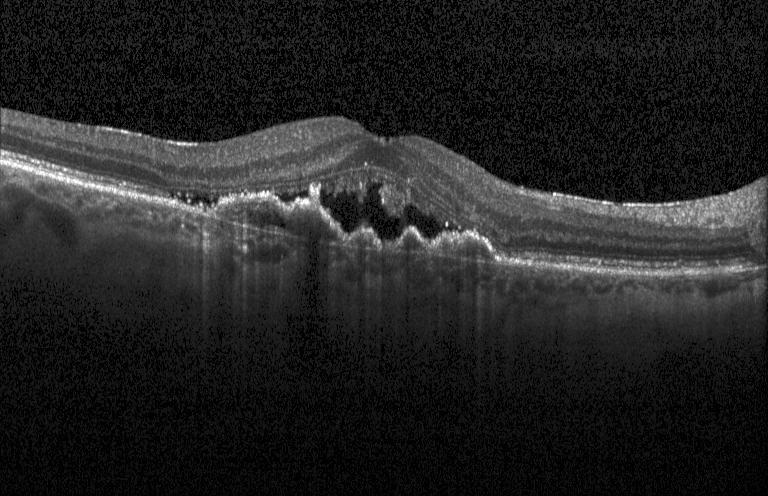 Retinal OCT B-scan — Assessment: a choroidal neovascular membrane.